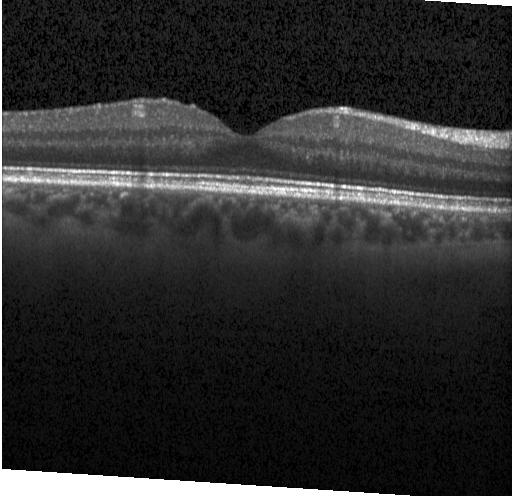 Retinal OCT B-scan
OCT finding: no choroidal neovascularization, no diabetic macular edema, and no drusen.